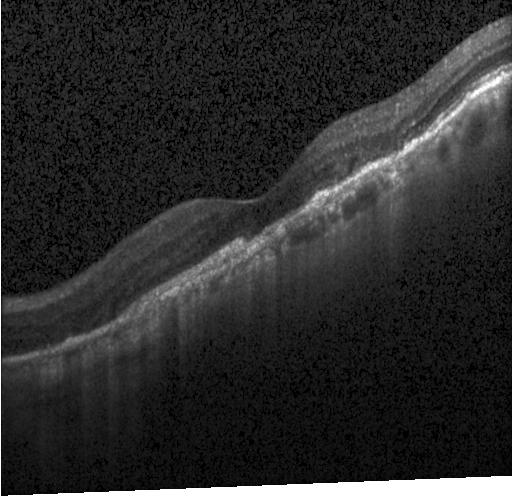
Retinal OCT cross-section · acquired on a Heidelberg Spectralis · macular scan — The scan shows a choroidal neovascular membrane.